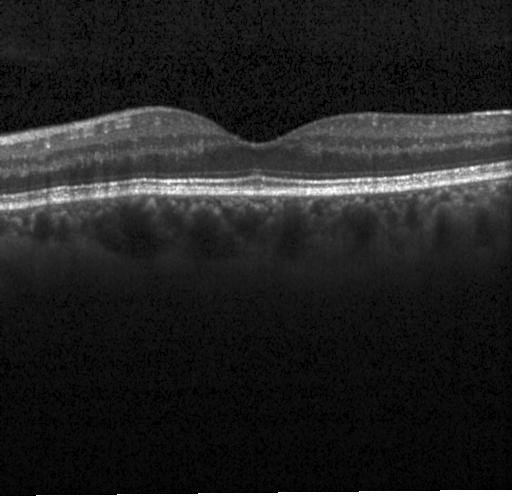

Spectral-domain OCT B-scan: no choroidal neovascularization, no diabetic macular edema, and no drusen.